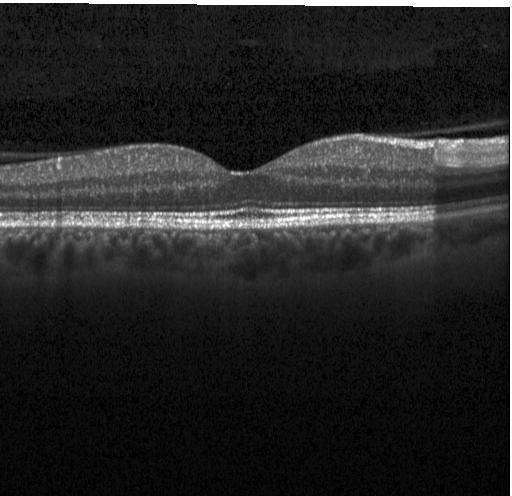

Fovea-centered, retinal OCT cross-section, spectral-domain optical coherence tomography, acquired on a Heidelberg Spectralis.
No choroidal neovascularization, diabetic macular edema, or drusen.